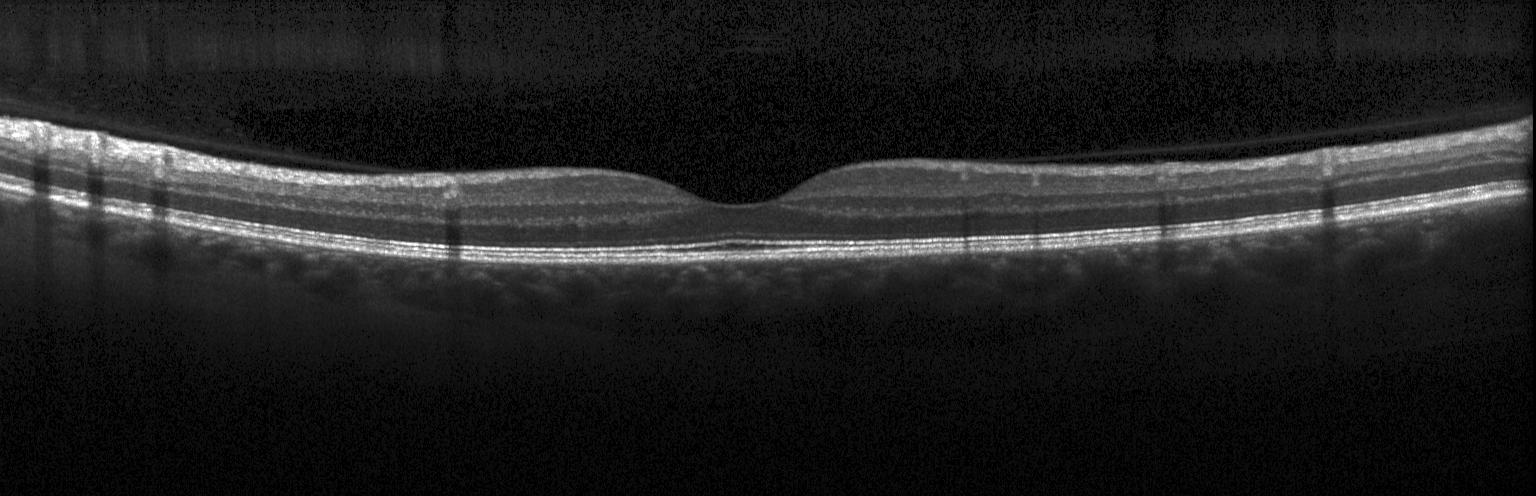

SD-OCT, centered on the fovea, optical coherence tomography B-scan. Assessment: no CNV, DME, or drusen.